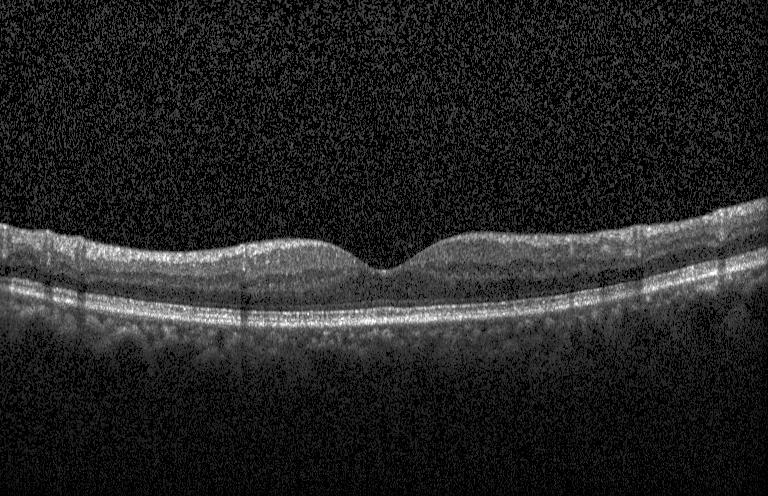
Spectral-domain OCT · Heidelberg Spectralis · OCT line scan
Dx: no evidence of CNV, DME, or drusen.